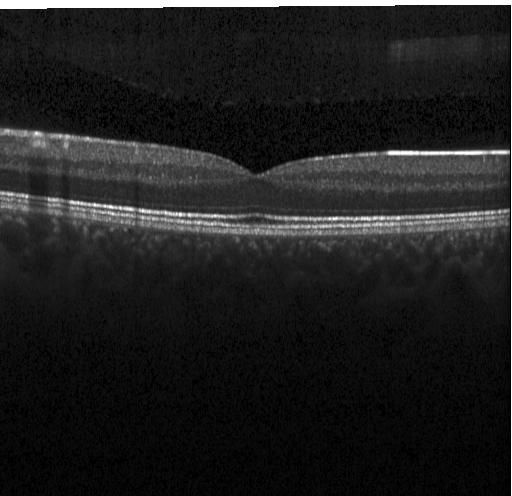

Impression: no evidence of choroidal neovascularization, diabetic macular edema, or drusen.